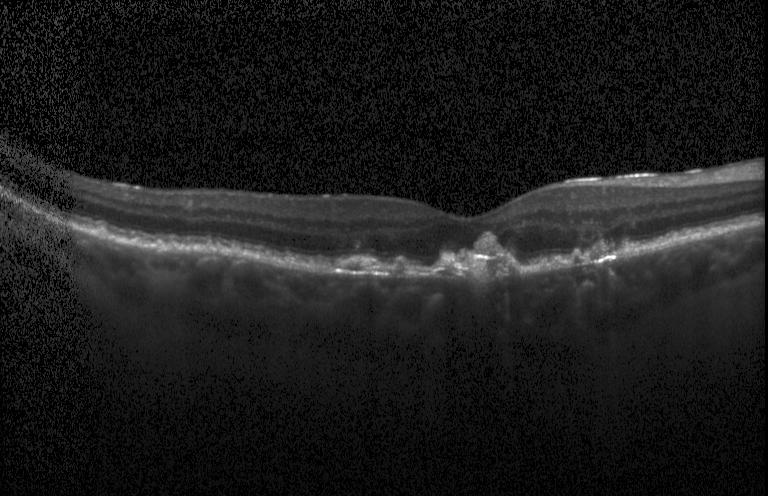

OCT line scan
This B-scan demonstrates a choroidal neovascular membrane.